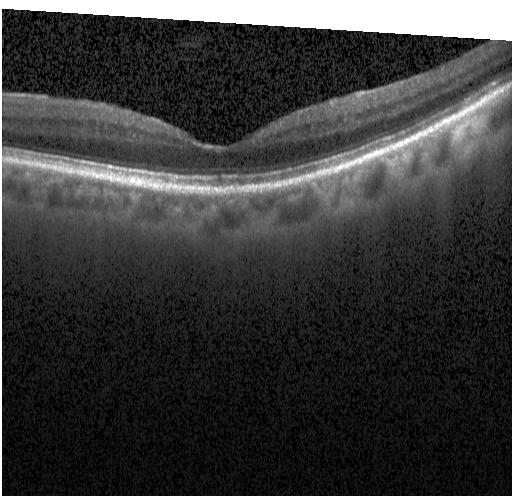
Optical coherence tomography B-scan · spectral-domain optical coherence tomography. Macular OCT: no evidence of choroidal neovascularization, diabetic macular edema, or drusen.